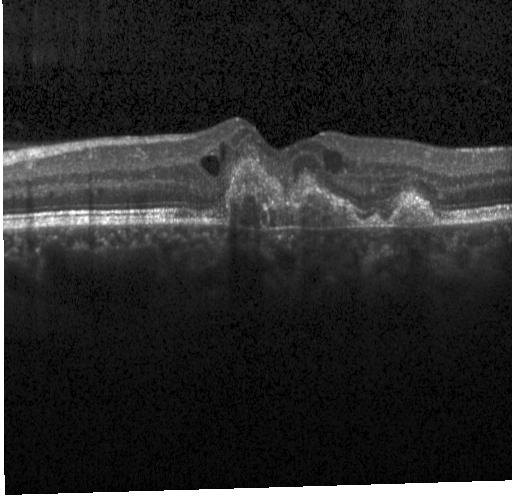

Spectral-domain optical coherence tomography. Retinal OCT B-scan — Diagnosis: choroidal neovascularization (CNV).